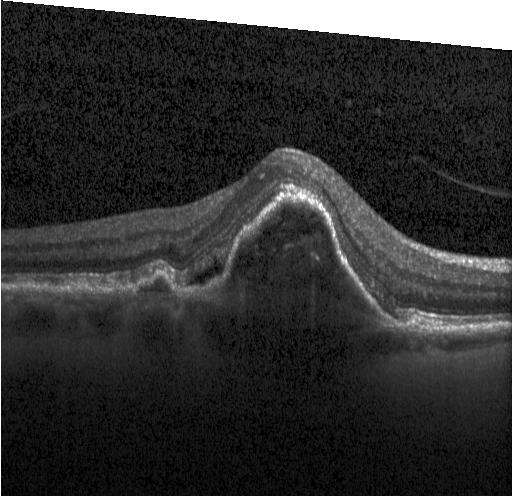

Finding: choroidal neovascularization (CNV).